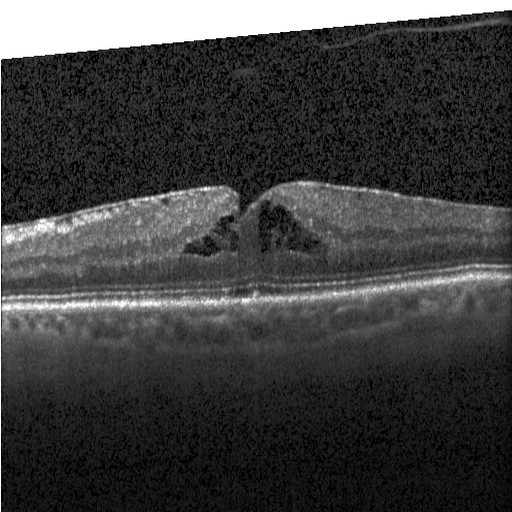
OCT line scan; horizontal scan through the fovea. OCT finding: diabetic macular edema.